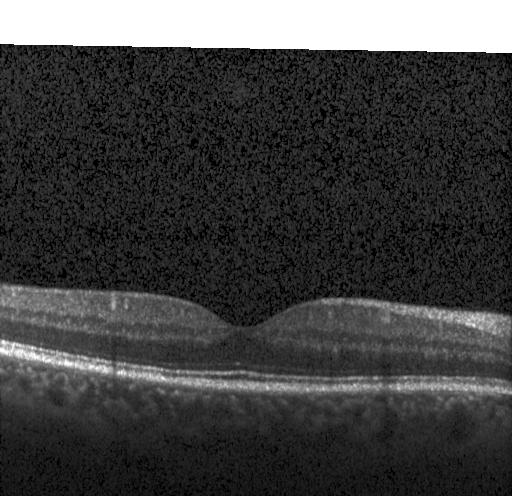 Fovea-centered. SD-OCT. OCT B-scan. Instrument: Heidelberg Spectralis.
Macular OCT: no choroidal neovascularization, no diabetic macular edema, and no drusen.